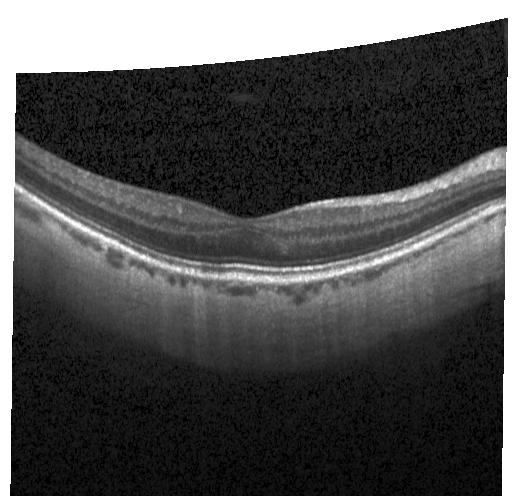 Dx: no choroidal neovascularization, diabetic macular edema, or drusen.